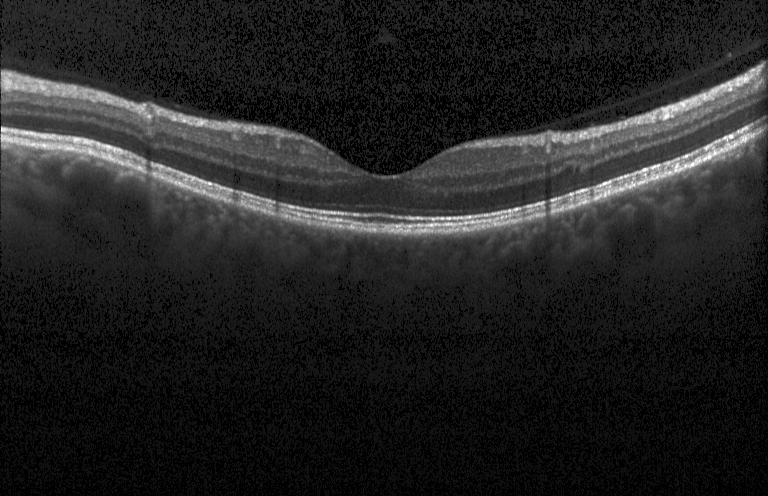
Retinal OCT B-scan. Horizontal scan through the fovea
Diagnosis: no evidence of choroidal neovascularization, diabetic macular edema, or drusen.